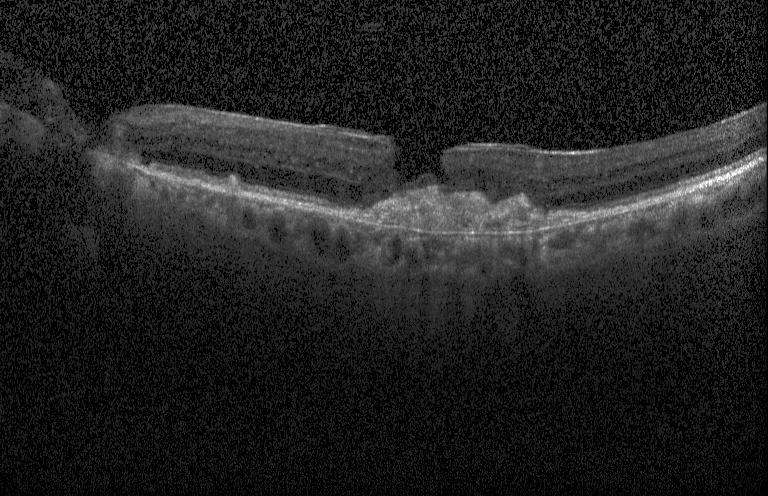

Finding: choroidal neovascularization (CNV).